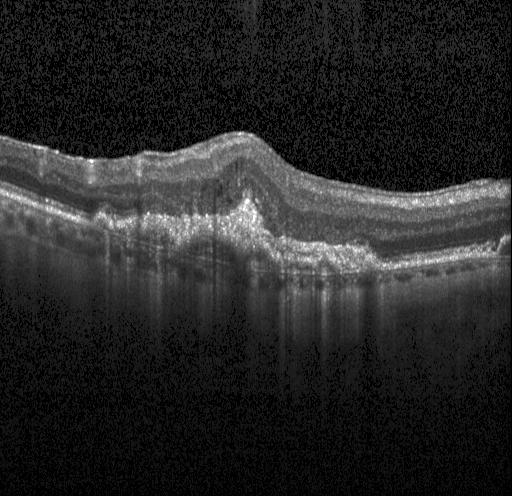

Spectral-domain OCT B-scan: choroidal neovascularization (CNV).